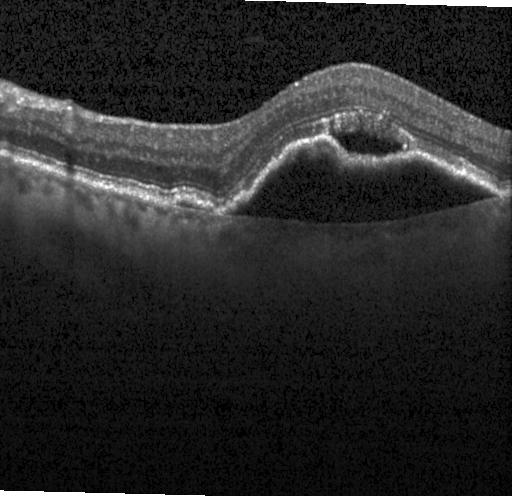 Macular OCT: a choroidal neovascular membrane.